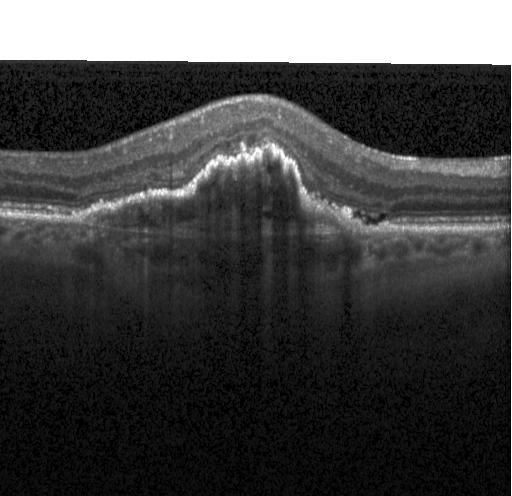

Diagnosis: a choroidal neovascular membrane.